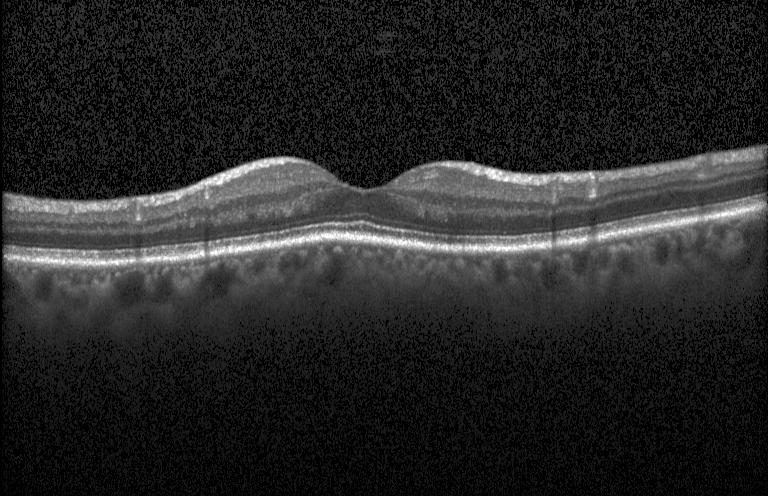
OCT scan showing neither choroidal neovascularization, diabetic macular edema, nor drusen.